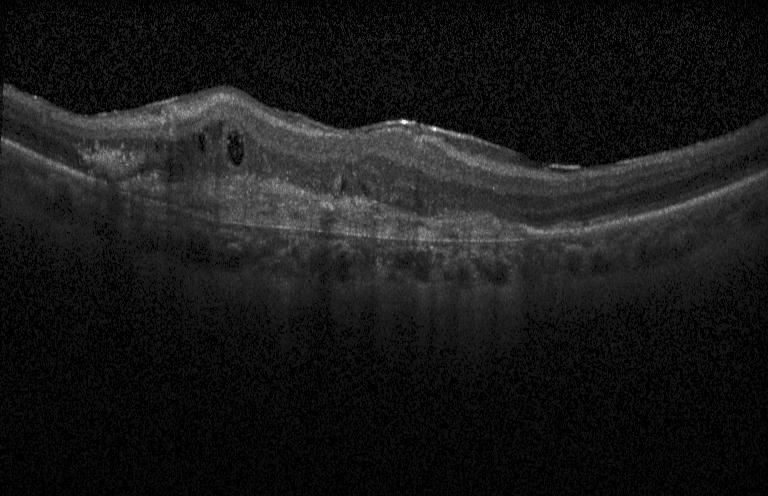
Dx: CNV.